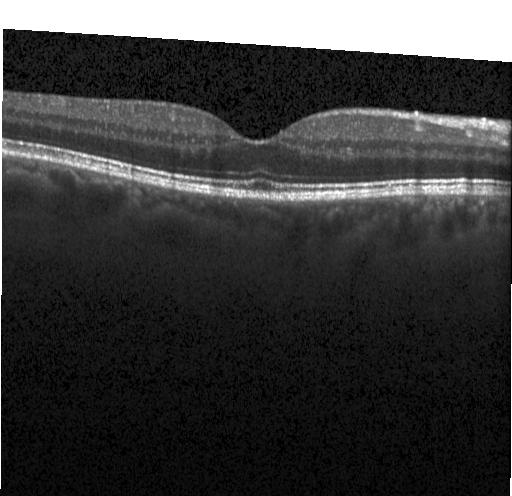
Heidelberg Spectralis, retinal OCT B-scan
No CNV, DME, or drusen.